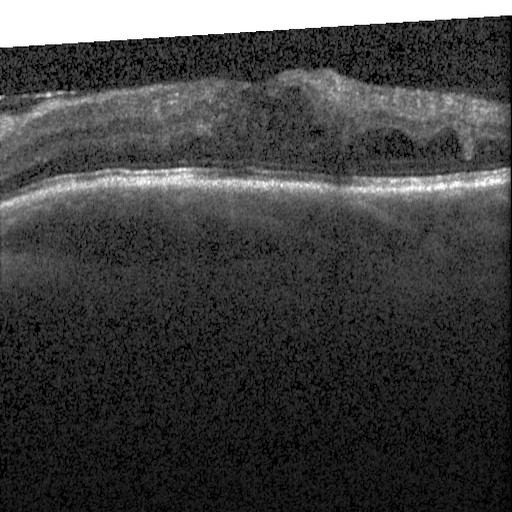

Spectral-domain OCT, through the macula, OCT B-scan, acquired on a Heidelberg Spectralis. Finding: diabetic macular edema (DME).